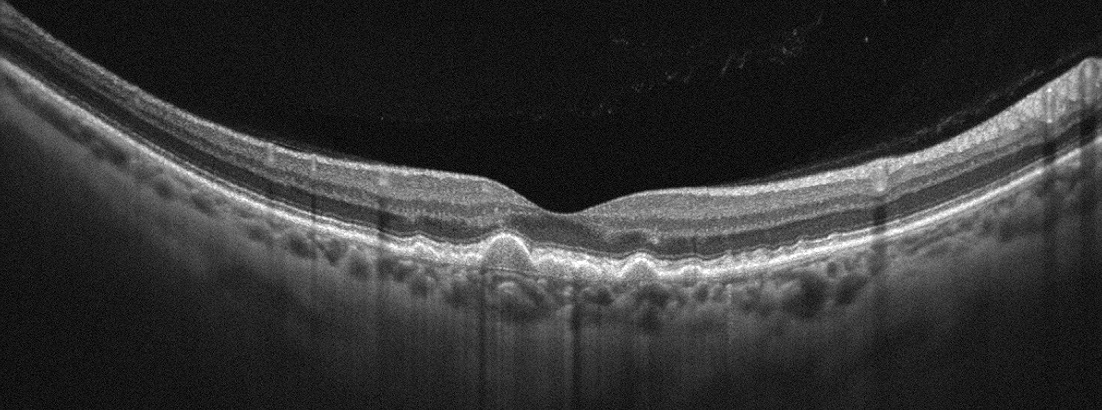

OCT line scan — Impression: age-related macular degeneration (AMD).